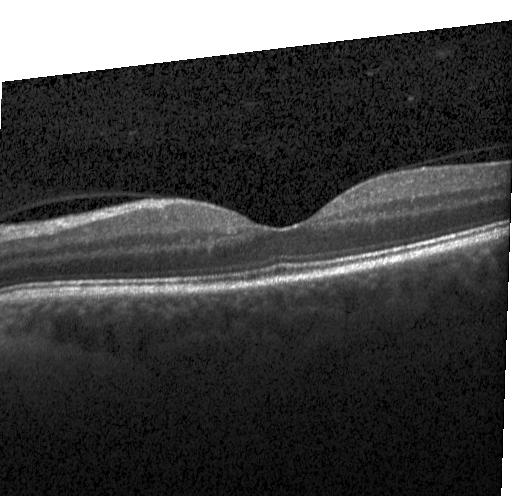

Spectral-domain optical coherence tomography. Heidelberg Spectralis. Horizontal scan through the fovea. Optical coherence tomography B-scan — This B-scan demonstrates neither choroidal neovascularization, diabetic macular edema, nor drusen.